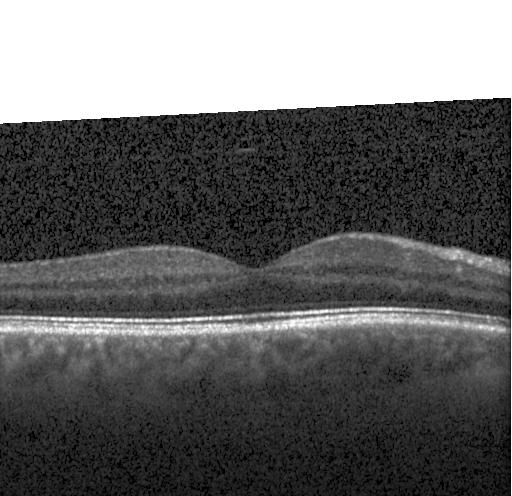 OCT line scan; SD-OCT — Neither choroidal neovascularization, diabetic macular edema, nor drusen.